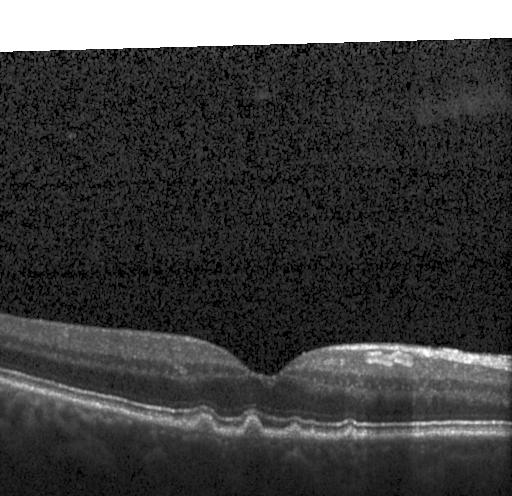

Heidelberg Spectralis OCT system, spectral-domain OCT, retinal OCT B-scan, centered on the fovea.
Impression: drusen.